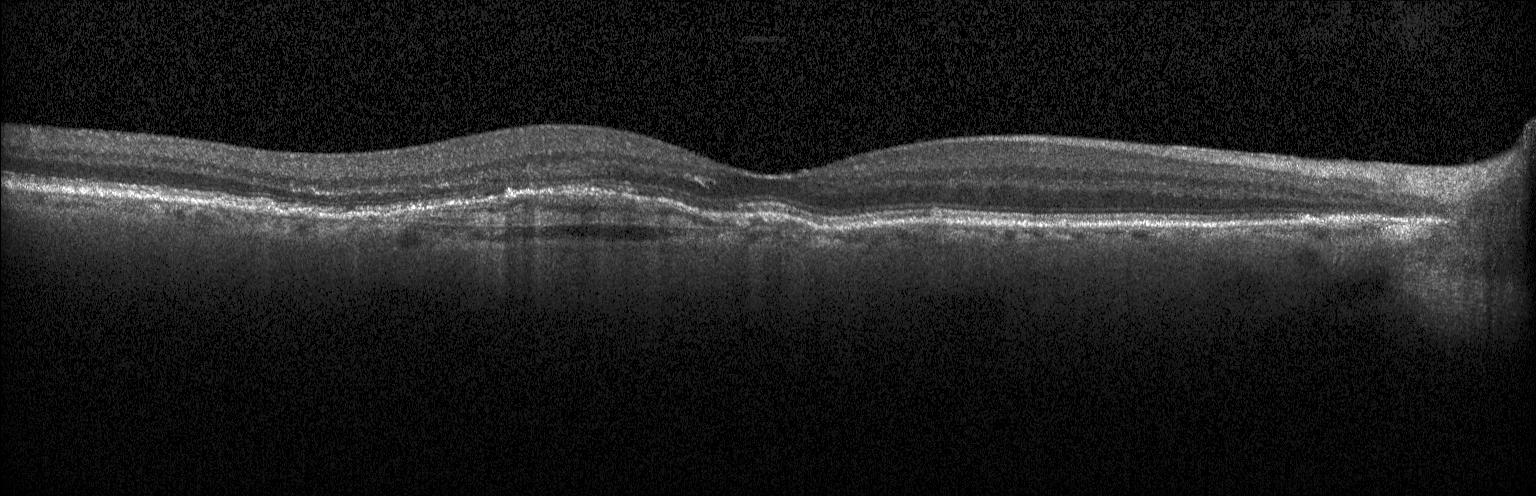

Acquired on a Heidelberg Spectralis · fovea-centered · retinal OCT B-scan — Dx: a choroidal neovascular membrane.